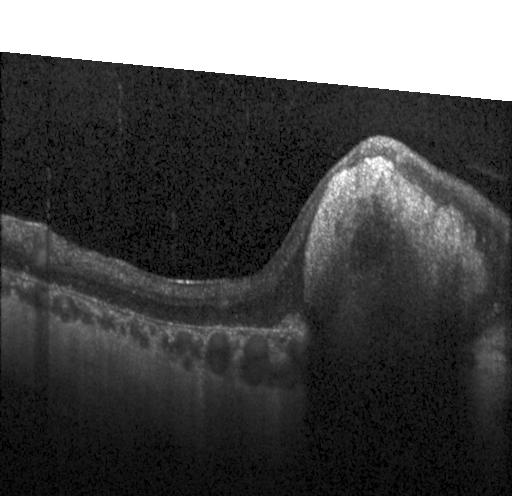
Impression: a choroidal neovascular membrane.